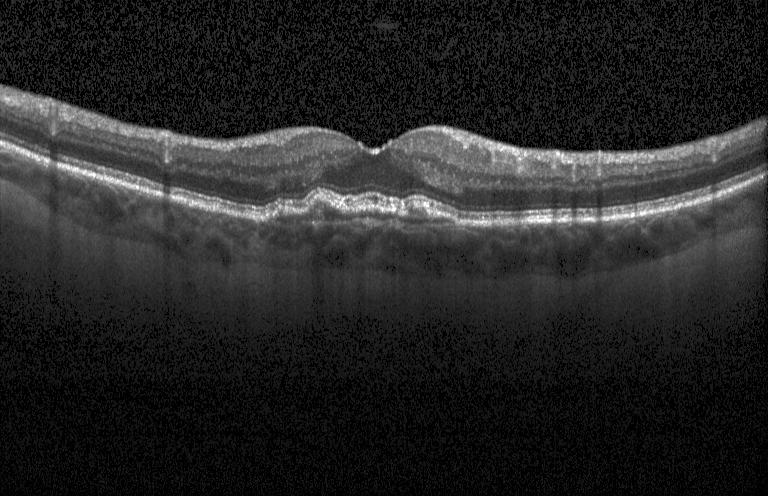 Spectral-domain OCT · through the macula · OCT B-scan · Heidelberg Spectralis OCT system.
Diagnosis: choroidal neovascularization (CNV).